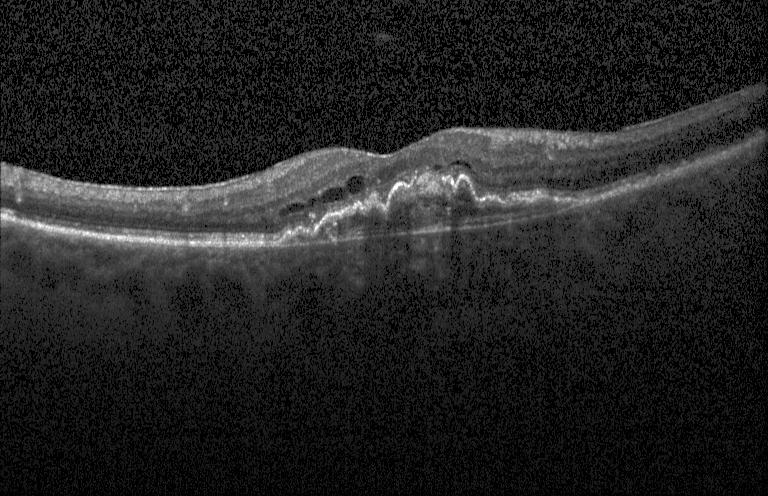

Impression: a choroidal neovascular membrane.